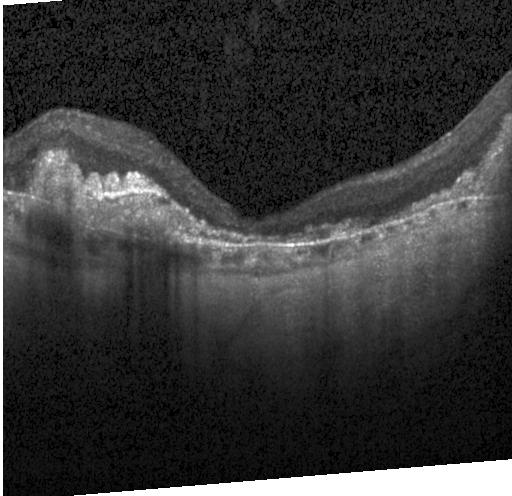

Optical coherence tomography B-scan, fovea-centered, spectral-domain optical coherence tomography. OCT finding: a choroidal neovascular membrane.